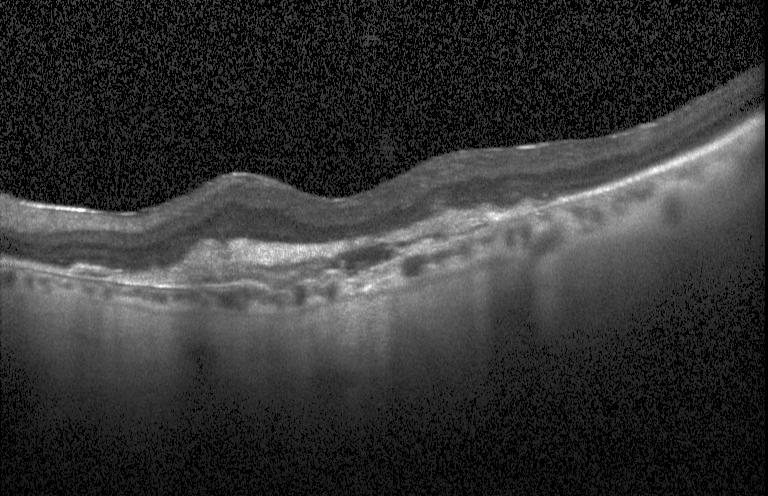
OCT scan showing CNV.